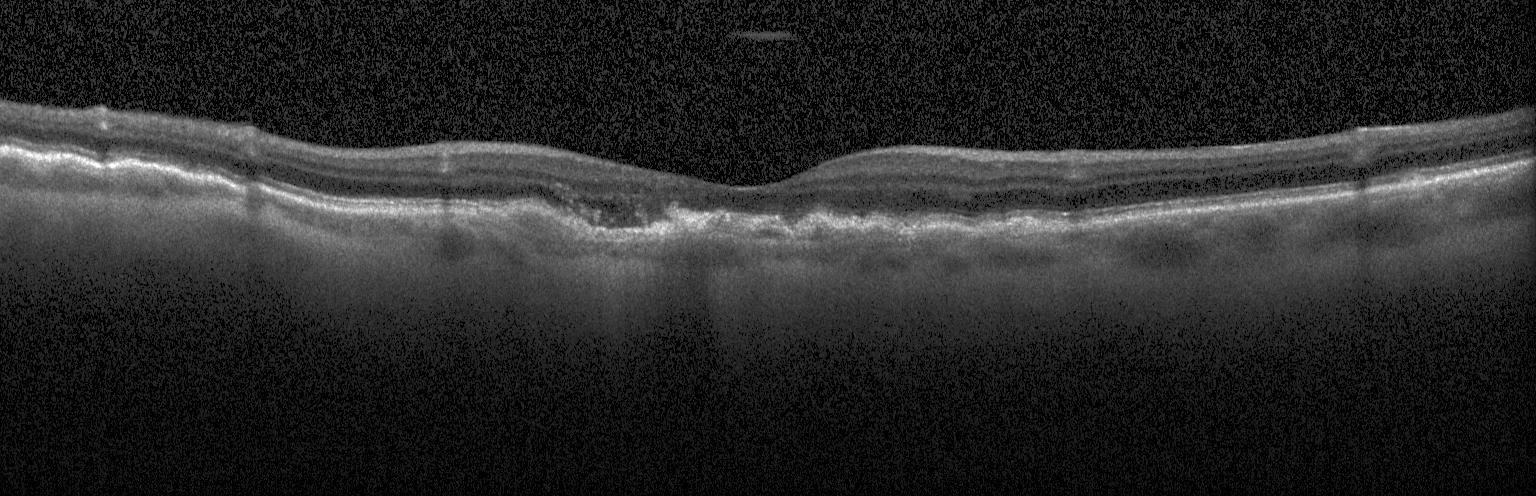

OCT line scan. Heidelberg Spectralis OCT system.
Dx: a choroidal neovascular membrane.